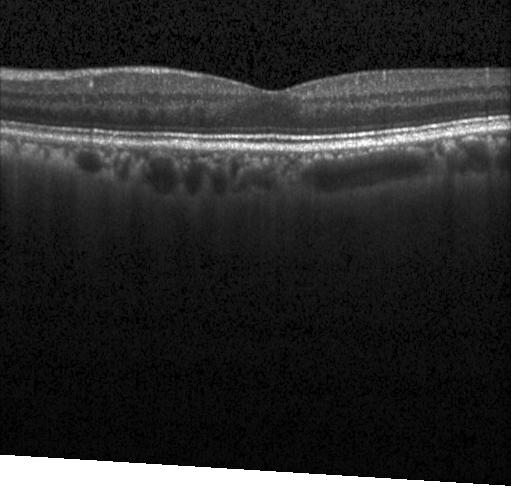 Assessment: neither CNV, DME, nor drusen.